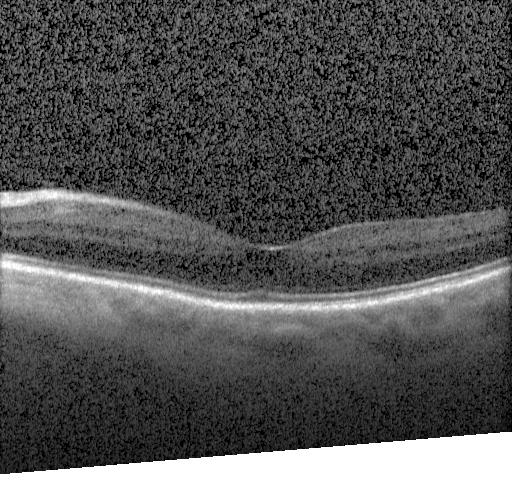
Heidelberg Spectralis, optical coherence tomography B-scan, spectral-domain OCT — No evidence of choroidal neovascularization, diabetic macular edema, or drusen.